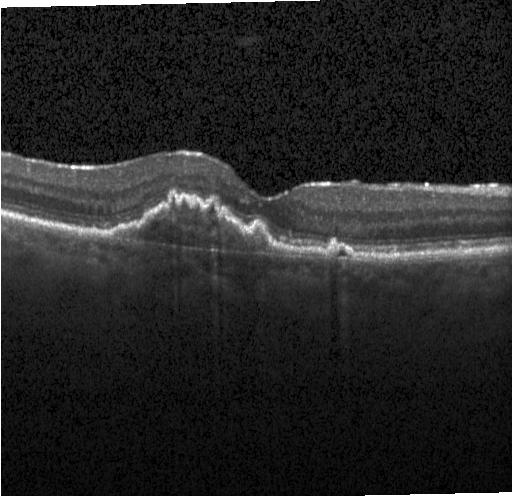 This B-scan demonstrates choroidal neovascularization.